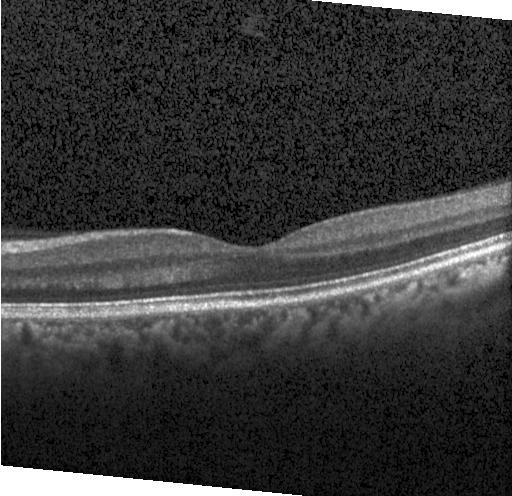
Through the macula; optical coherence tomography scan
Finding: neither CNV, DME, nor drusen.